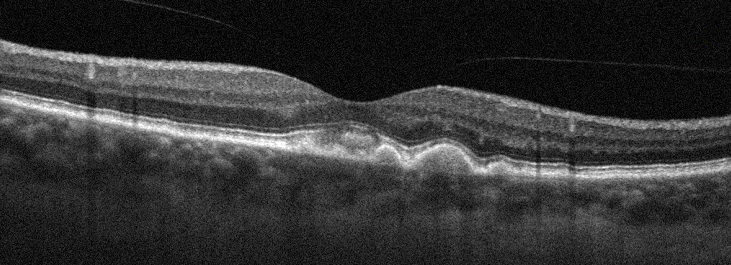
Instrument: Optovue Avanti RTVue XR · optical coherence tomography B-scan
Impression: AMD.